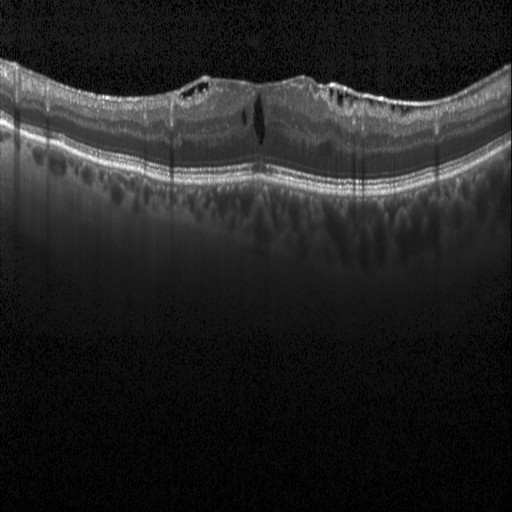
Heidelberg Spectralis OCT system · spectral-domain optical coherence tomography · OCT B-scan.
Dx: diabetic macular edema (DME).